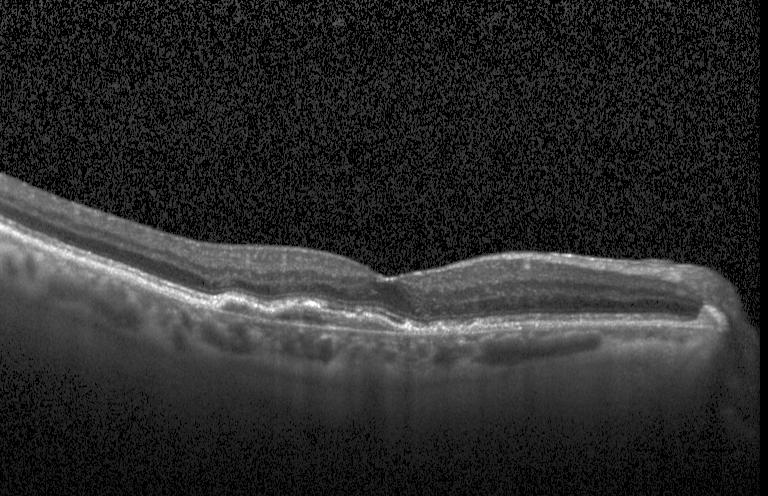
Dx: choroidal neovascularization.